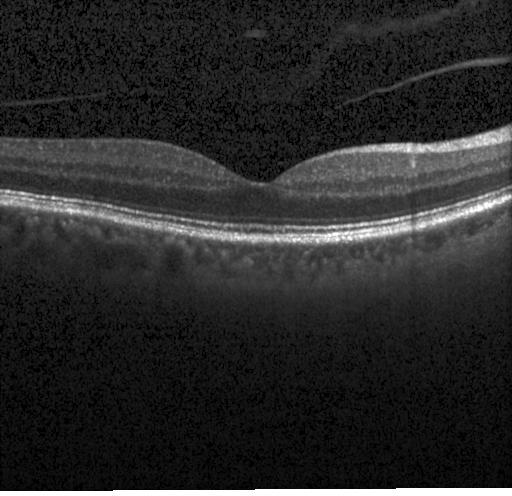 Through the macula · Heidelberg Spectralis OCT system · OCT B-scan · spectral-domain optical coherence tomography — Impression: no CNV, DME, or drusen.